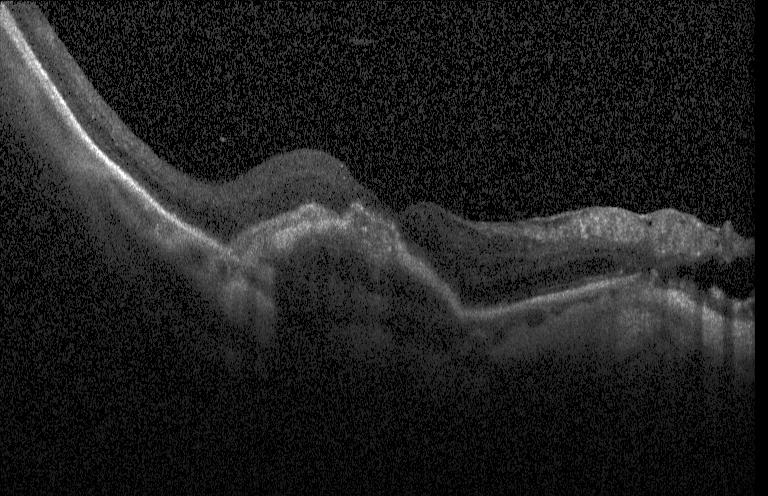 Spectral-domain OCT B-scan: a choroidal neovascular membrane.